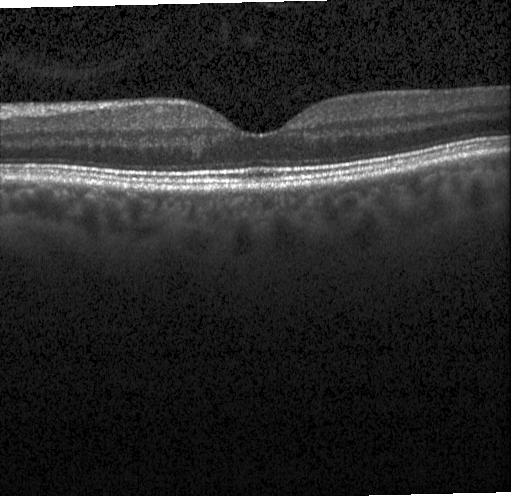

OCT scan showing no CNV, no DME, and no drusen.